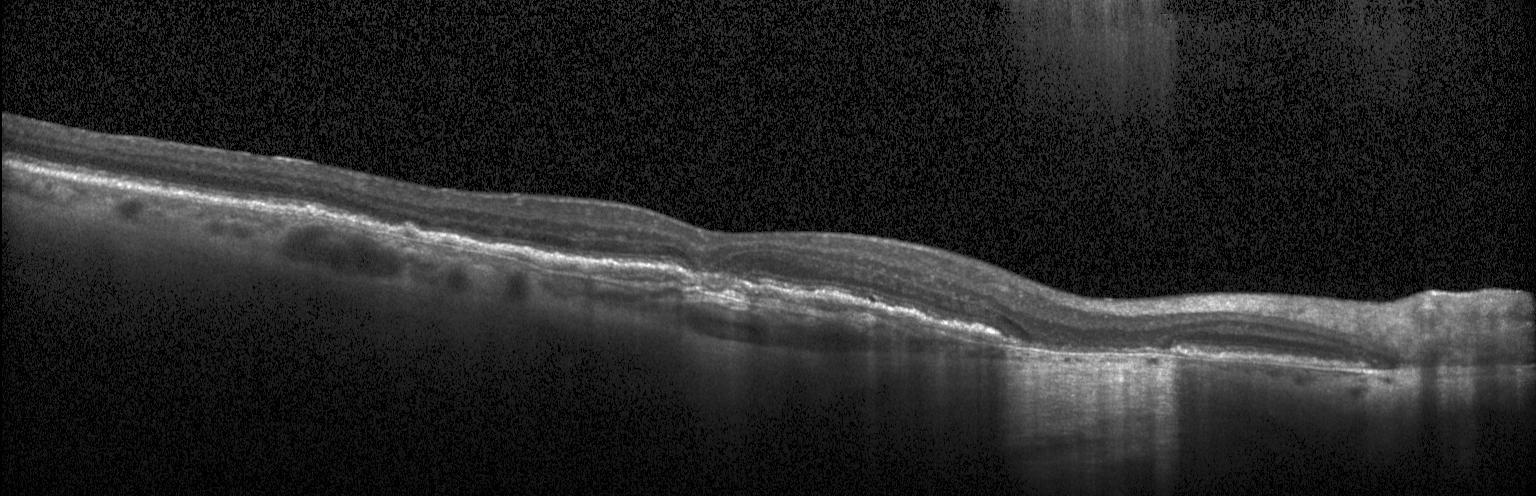

Finding: a choroidal neovascular membrane.